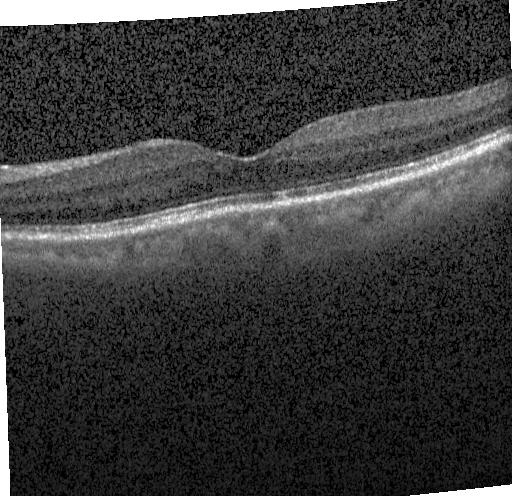

This B-scan demonstrates no choroidal neovascularization, no diabetic macular edema, and no drusen.